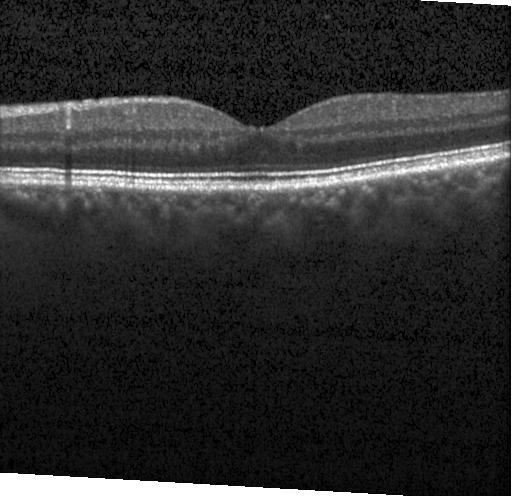

OCT B-scan, spectral-domain optical coherence tomography, horizontal scan through the fovea — Assessment: no evidence of choroidal neovascularization, diabetic macular edema, or drusen.